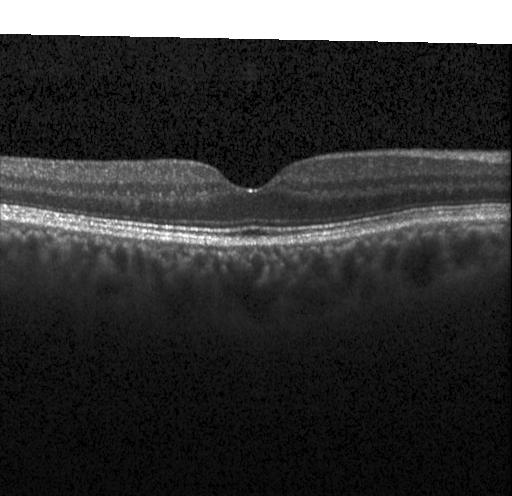
Instrument: Heidelberg Spectralis. Through the macula. SD-OCT. OCT B-scan
Finding: neither CNV, DME, nor drusen.